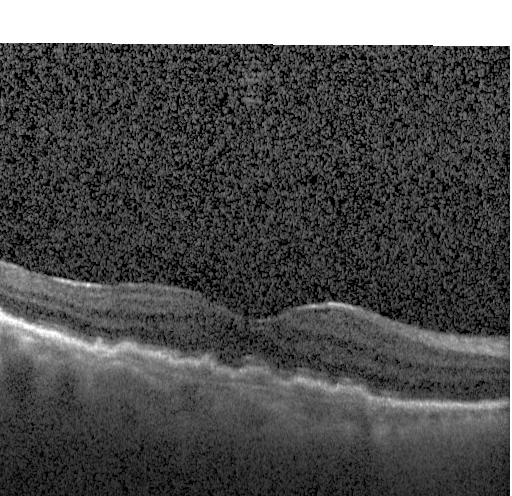 OCT line scan, spectral-domain optical coherence tomography. Choroidal neovascularization.